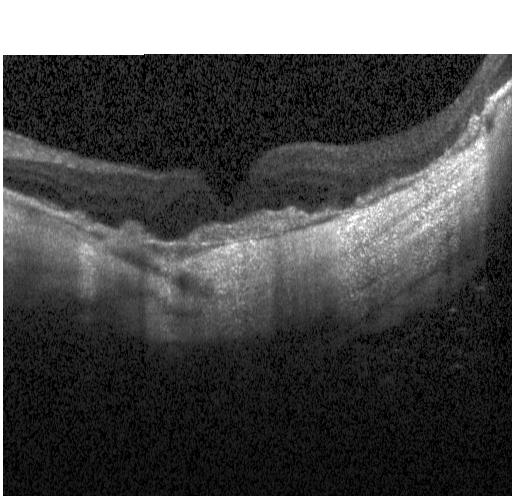 Macular OCT demonstrating CNV.